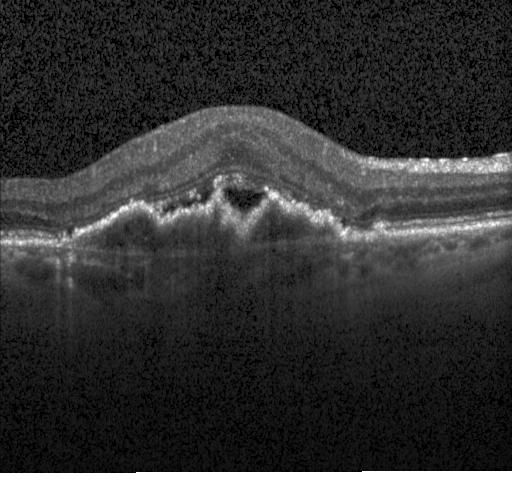
Instrument: Heidelberg Spectralis, OCT B-scan.
Finding: choroidal neovascularization (CNV).